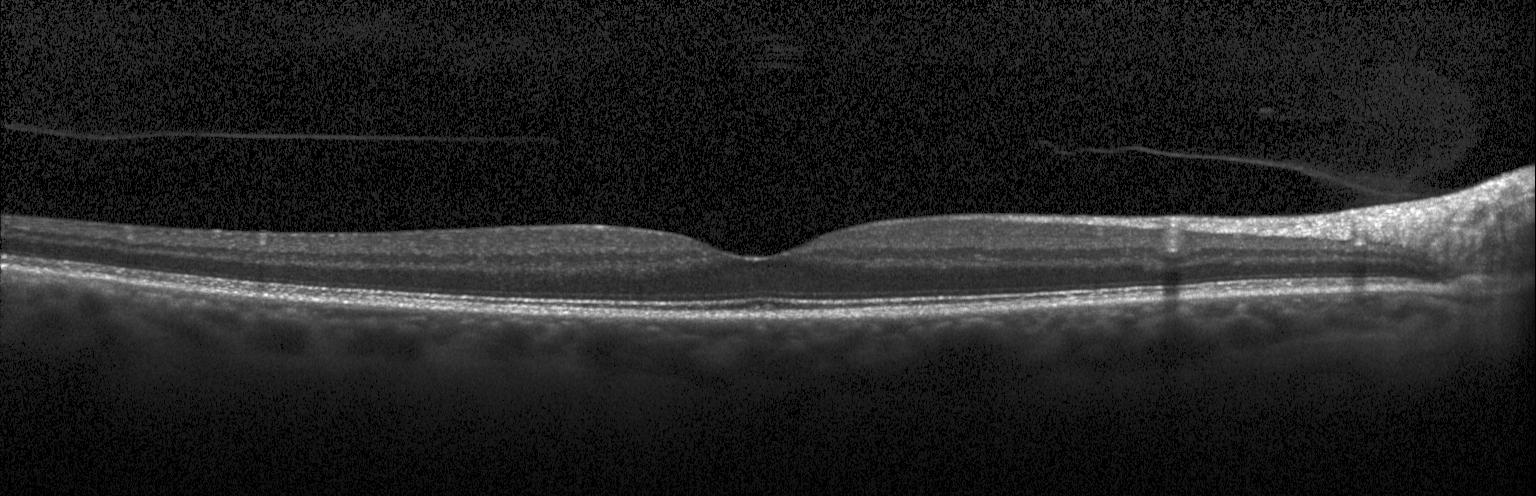
Finding: no choroidal neovascularization, diabetic macular edema, or drusen.